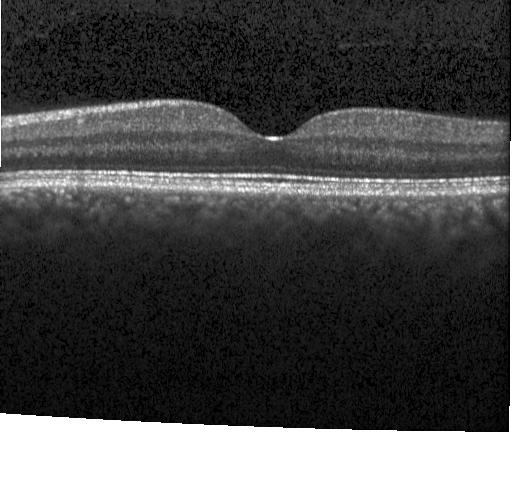 Retinal OCT B-scan
Finding: no choroidal neovascularization, no diabetic macular edema, and no drusen.